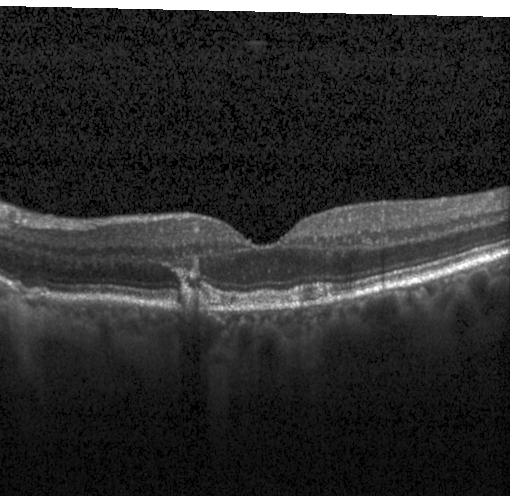
Heidelberg Spectralis OCT system · spectral-domain optical coherence tomography · retinal OCT B-scan.
OCT finding: multiple drusen.